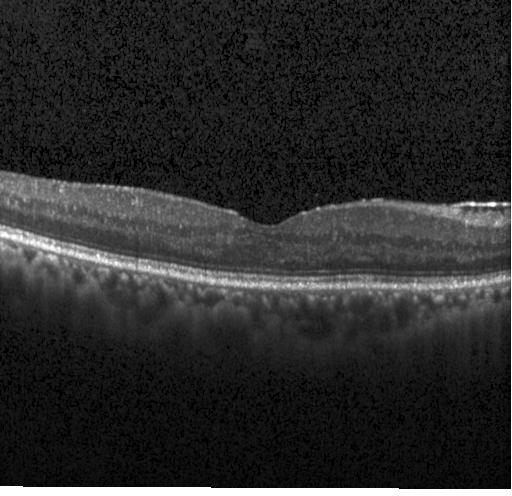
OCT B-scan showing no choroidal neovascularization, diabetic macular edema, or drusen.